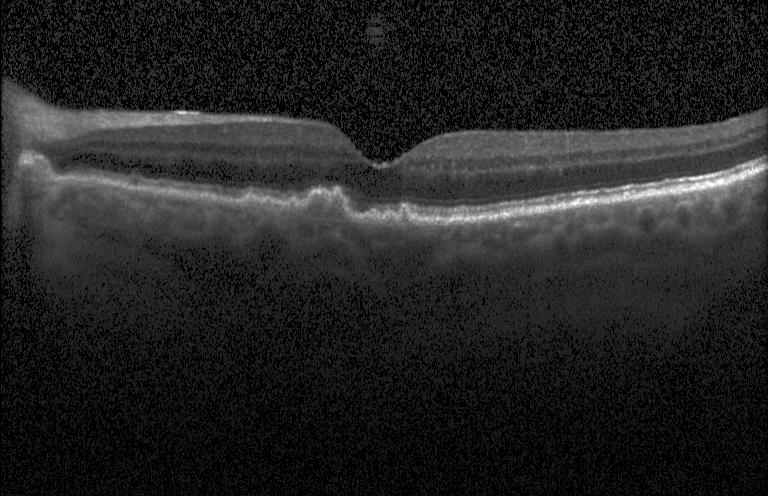
Optical coherence tomography scan — Dx: drusen.